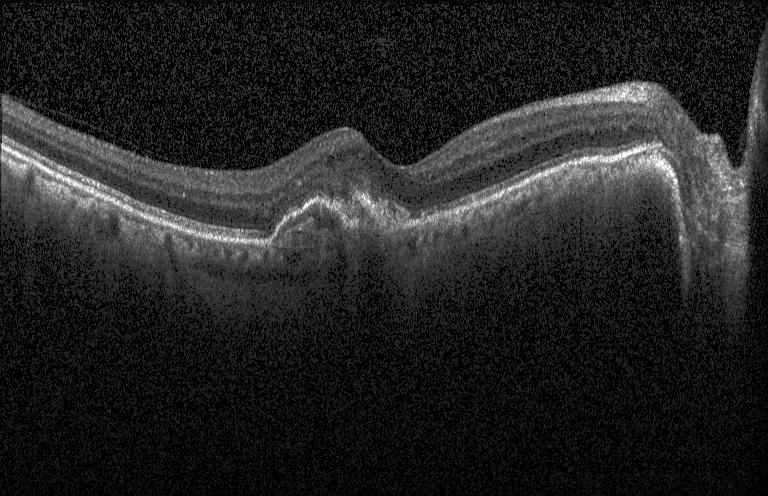

SD-OCT · Heidelberg Spectralis · retinal OCT B-scan. A choroidal neovascular membrane.